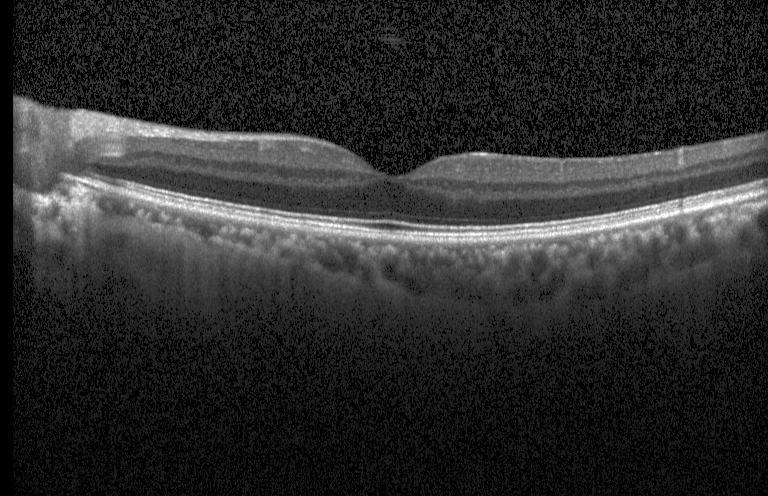 Horizontal scan through the fovea; optical coherence tomography B-scan — Diagnosis: no choroidal neovascularization, no diabetic macular edema, and no drusen.